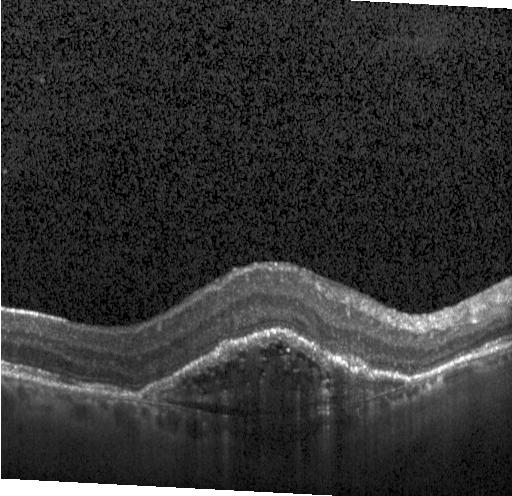

Spectral-domain optical coherence tomography. Retinal OCT B-scan. Horizontal scan through the fovea
Impression: a choroidal neovascular membrane.